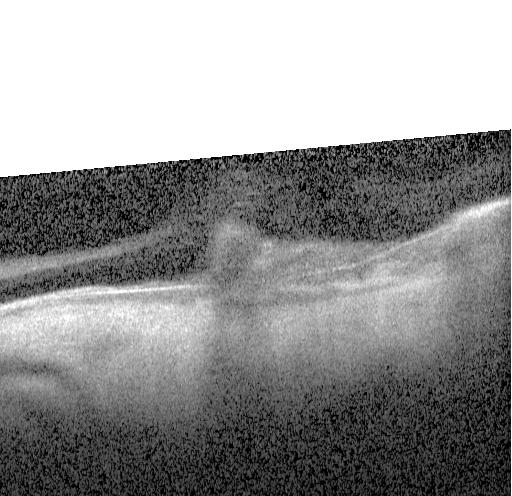 Through the macula; optical coherence tomography B-scan; Heidelberg Spectralis; spectral-domain optical coherence tomography.
Diagnosis: CNV.